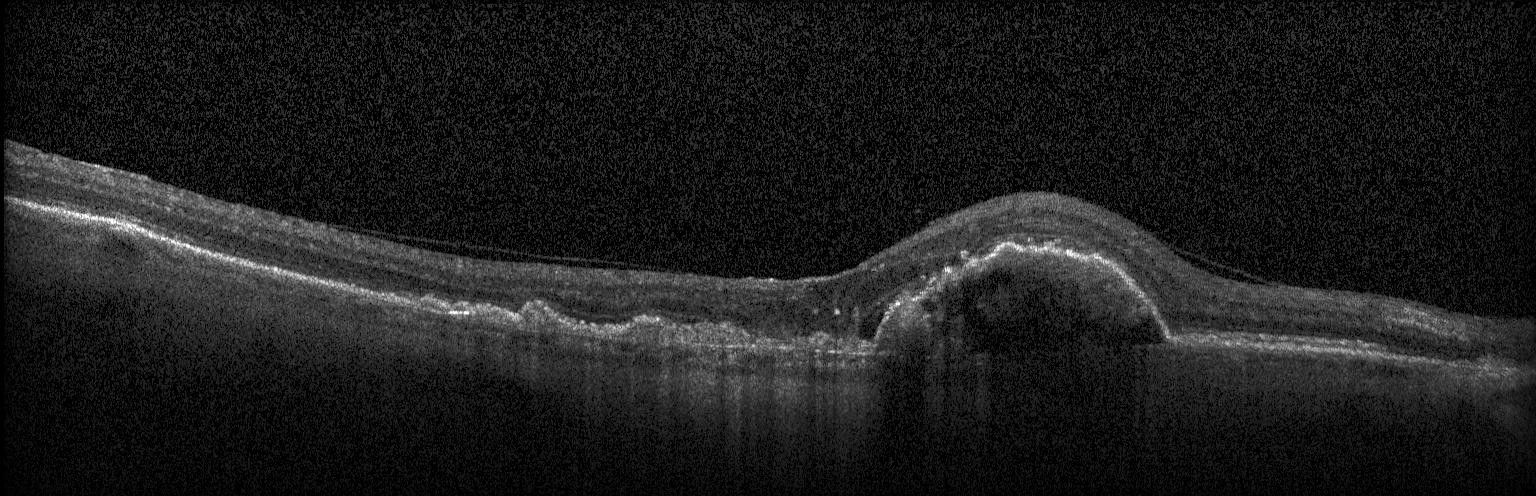
OCT finding: CNV.